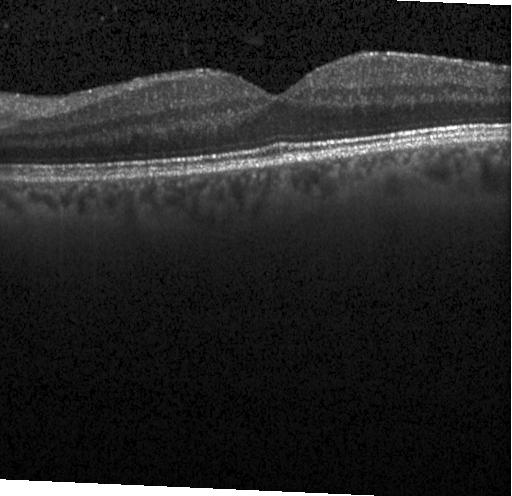 Optical coherence tomography scan
Impression: no choroidal neovascularization, no diabetic macular edema, and no drusen.